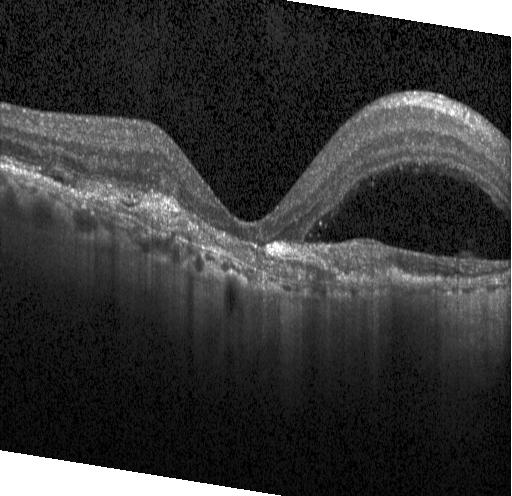
Impression: a choroidal neovascular membrane.